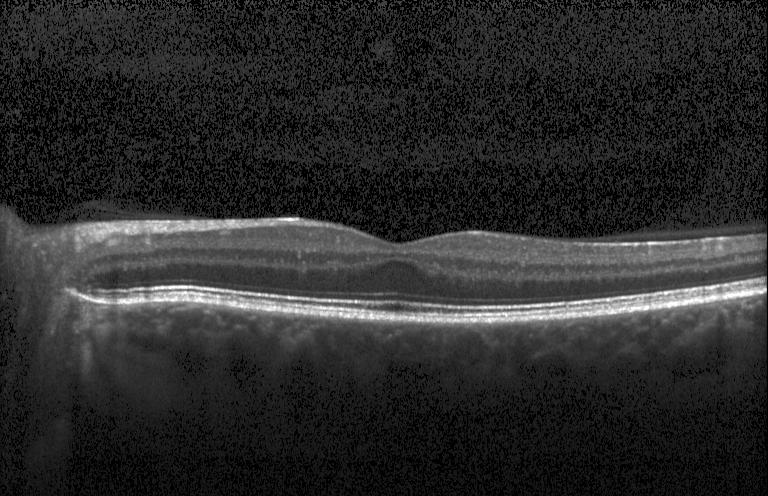
OCT scan showing no choroidal neovascularization, diabetic macular edema, or drusen.